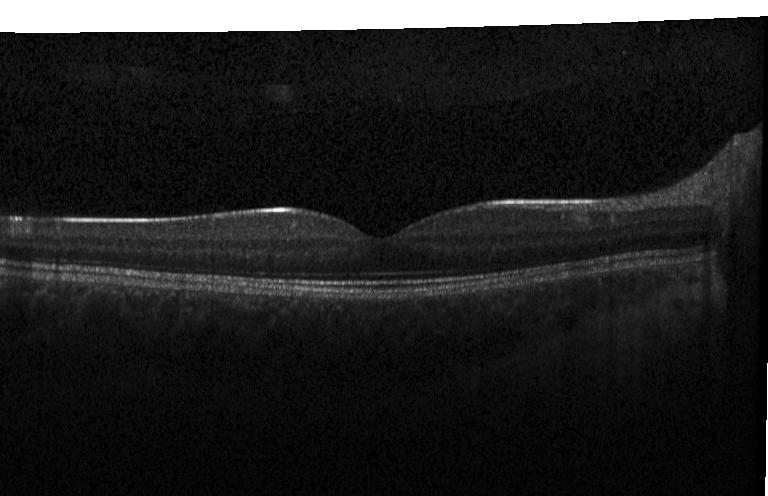
Acquired on a Heidelberg Spectralis; horizontal scan through the fovea; spectral-domain OCT; retinal OCT B-scan
Impression: no CNV, no DME, and no drusen.